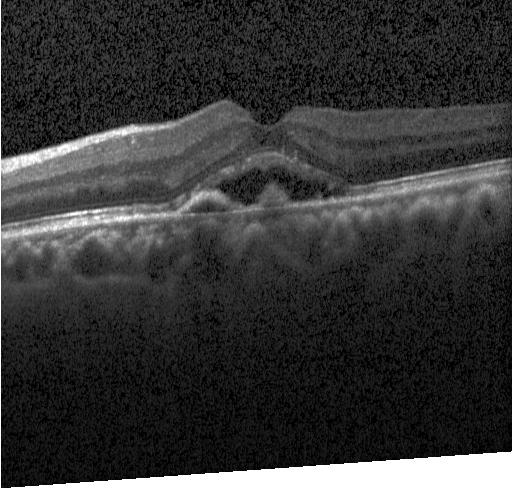 Centered on the fovea; optical coherence tomography B-scan. Choroidal neovascularization (CNV).